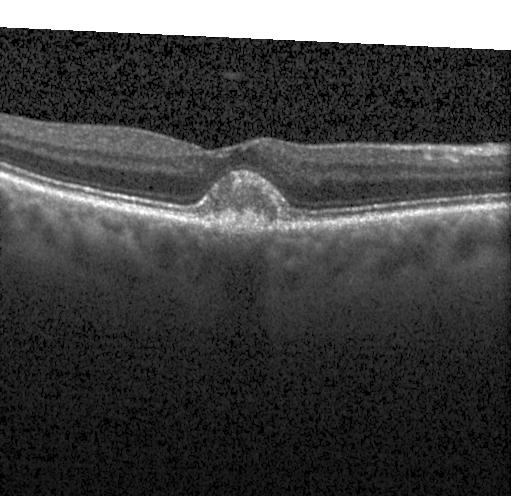 Retinal OCT B-scan. Spectral-domain optical coherence tomography. Instrument: Heidelberg Spectralis — Diagnosis: CNV.